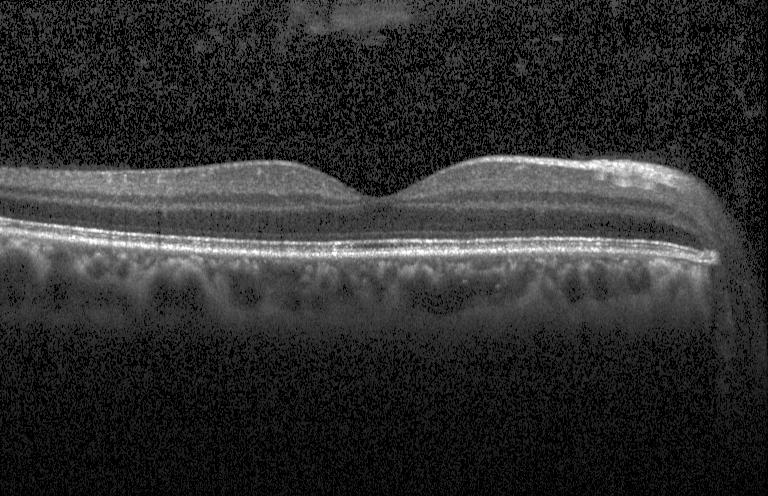 Retinal OCT cross-section showing neither choroidal neovascularization, diabetic macular edema, nor drusen.